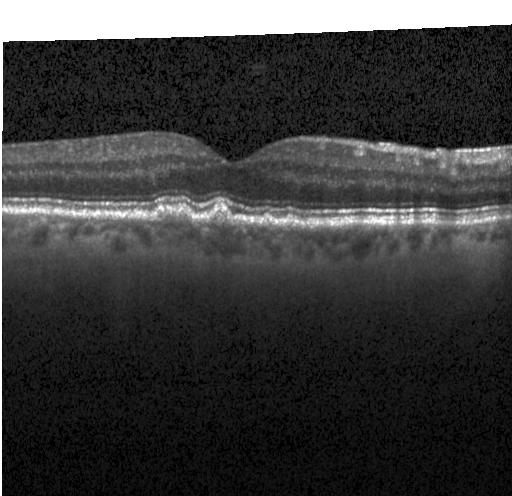 Retinal OCT cross-section — Impression: drusen.